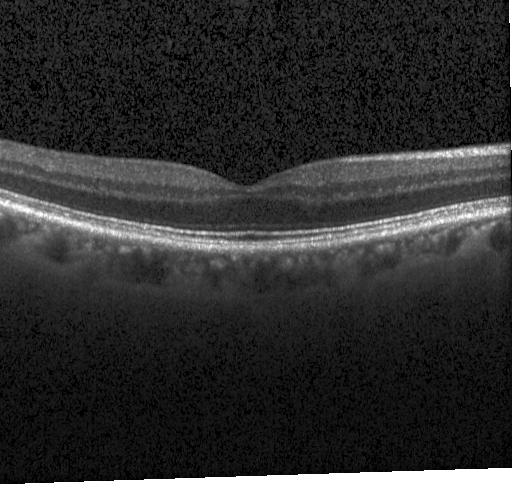

Finding: no CNV, DME, or drusen.